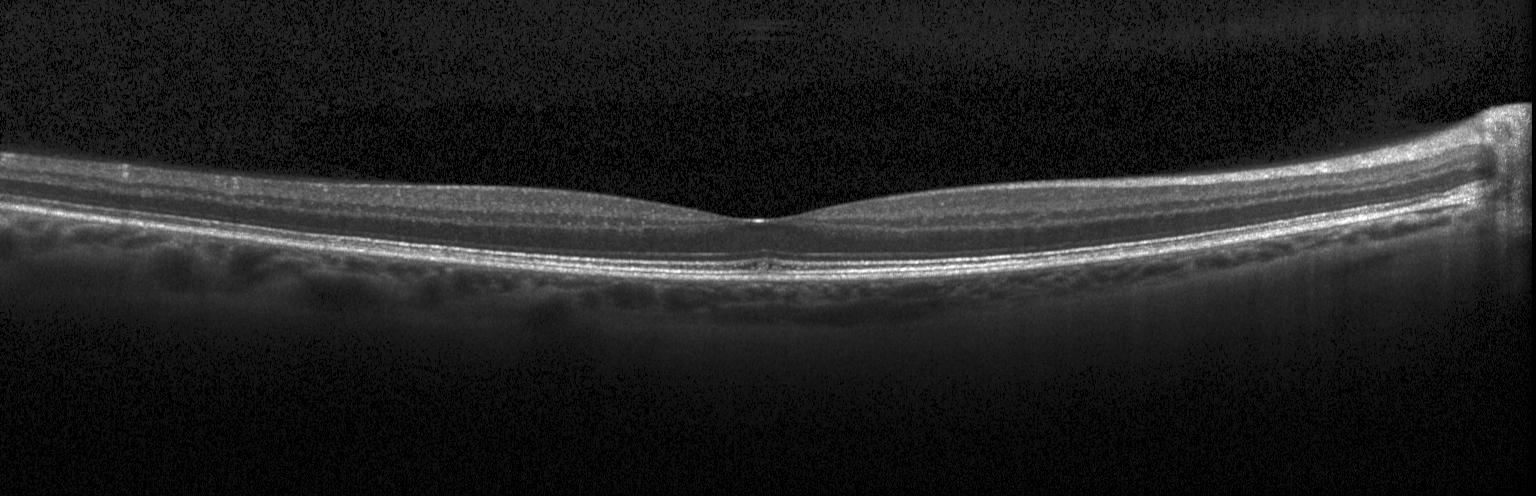

Instrument: Heidelberg Spectralis, retinal OCT cross-section, horizontal scan through the fovea
Assessment: neither CNV, DME, nor drusen.